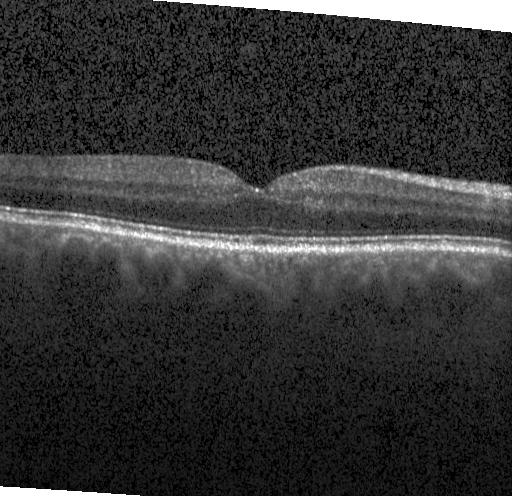 OCT B-scan, SD-OCT, Heidelberg Spectralis OCT system, through the macula — Finding: no choroidal neovascularization, diabetic macular edema, or drusen.